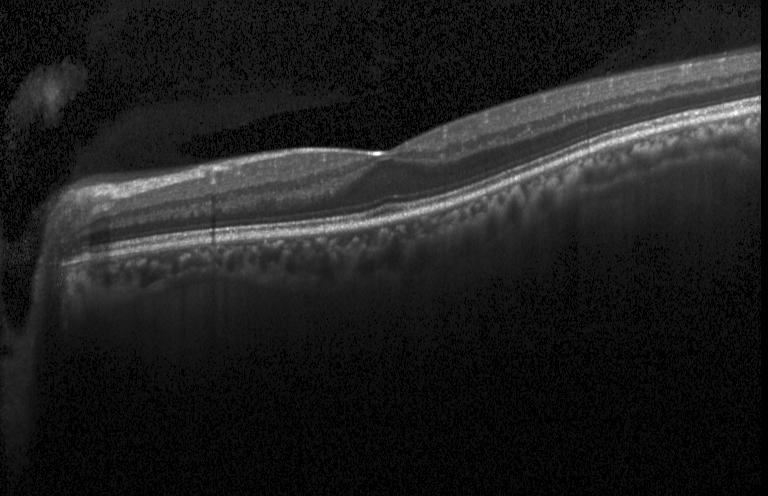

Retinal OCT B-scan · Heidelberg Spectralis OCT system · macular scan
Finding: neither CNV, DME, nor drusen.